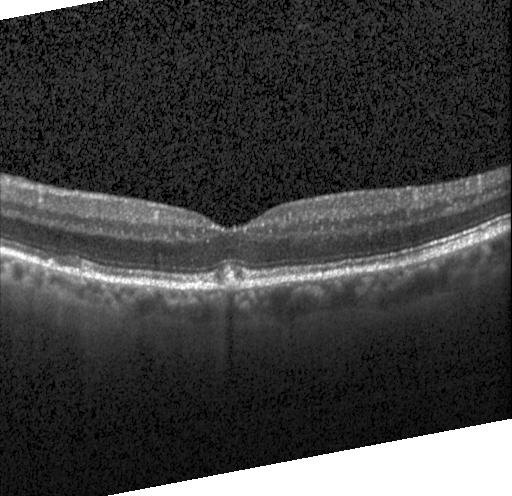 Assessment: drusen.